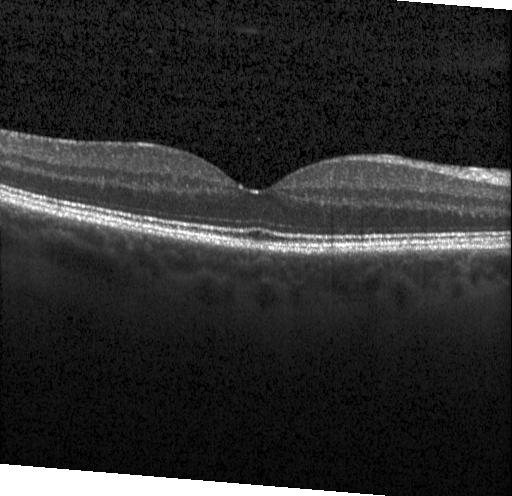
Impression: no choroidal neovascularization, diabetic macular edema, or drusen.